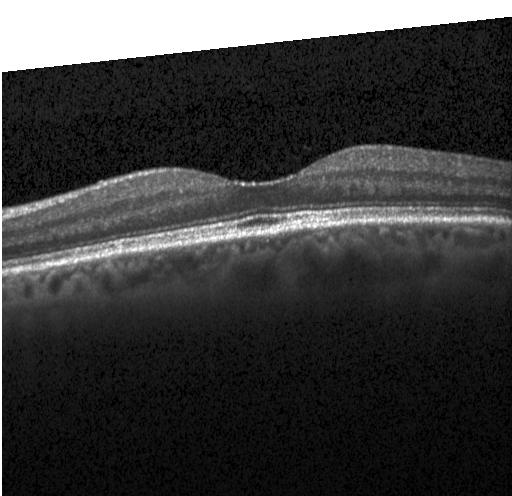 OCT scan showing no choroidal neovascularization, diabetic macular edema, or drusen.